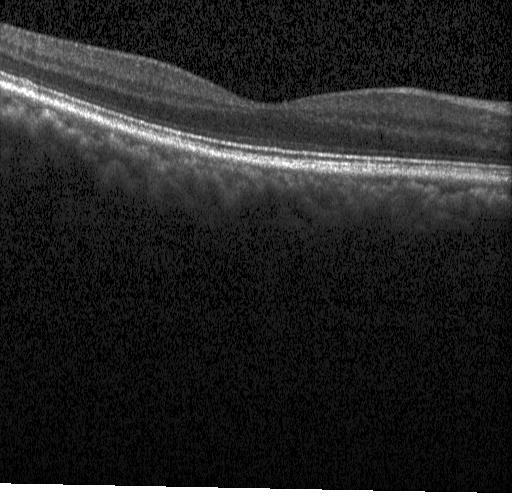
Retinal OCT cross-section
The scan shows no choroidal neovascularization, diabetic macular edema, or drusen.